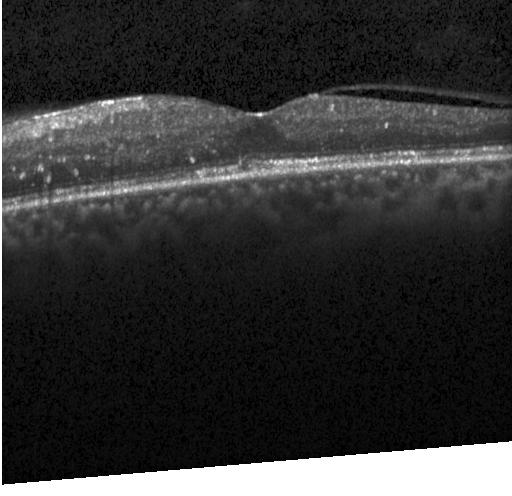 Acquired on a Heidelberg Spectralis. Optical coherence tomography B-scan. Centered on the fovea. Spectral-domain OCT
DME.